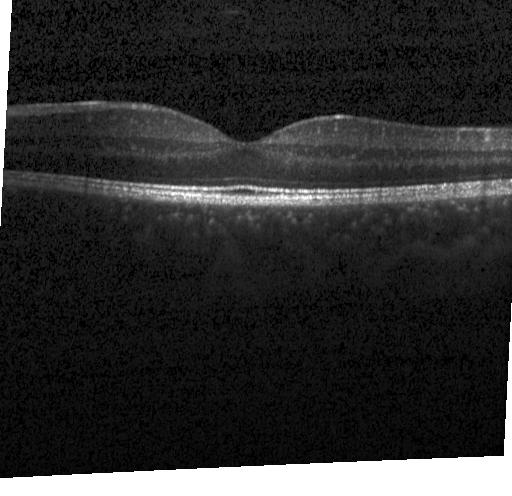 The scan shows no evidence of choroidal neovascularization, diabetic macular edema, or drusen.